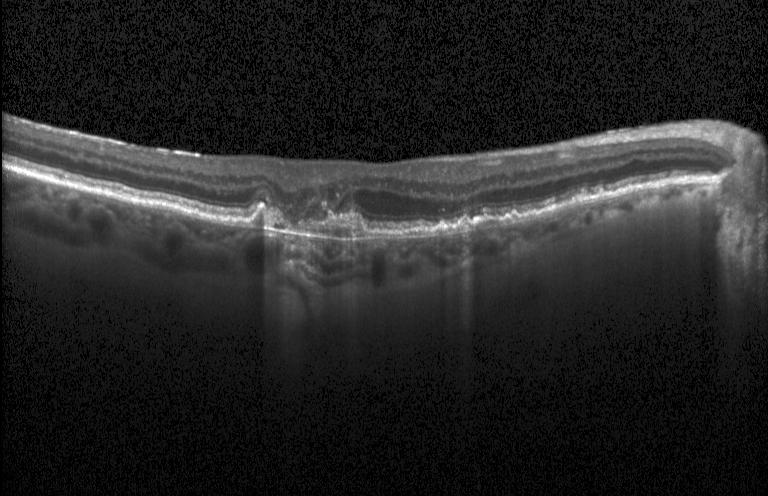 Heidelberg Spectralis OCT system · optical coherence tomography scan. Finding: CNV.